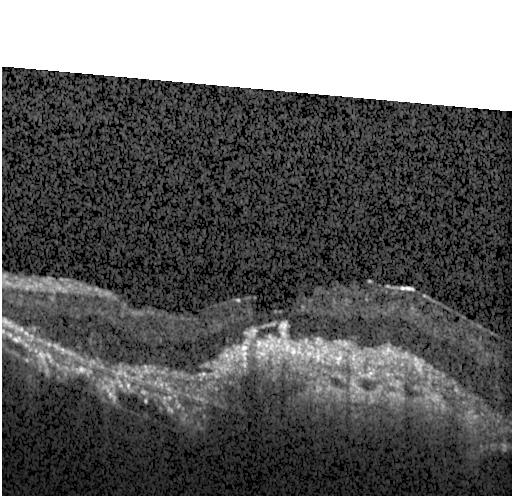

Instrument: Heidelberg Spectralis · macular scan · optical coherence tomography B-scan · spectral-domain optical coherence tomography — OCT finding: choroidal neovascularization (CNV).